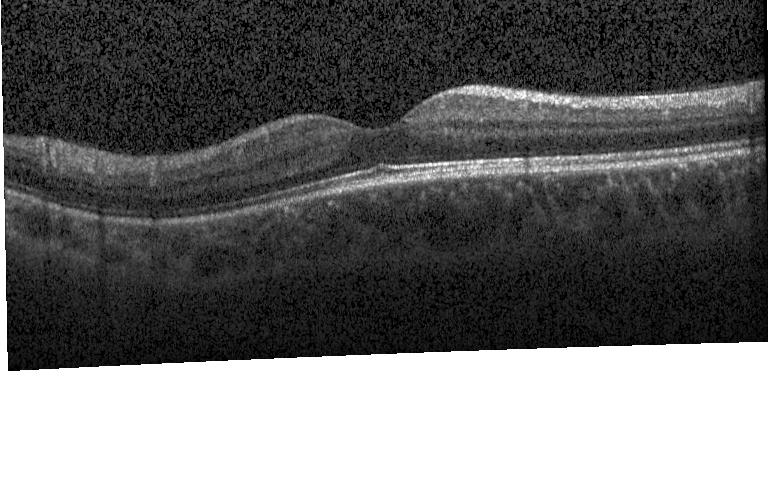
Impression: no CNV, no DME, and no drusen.